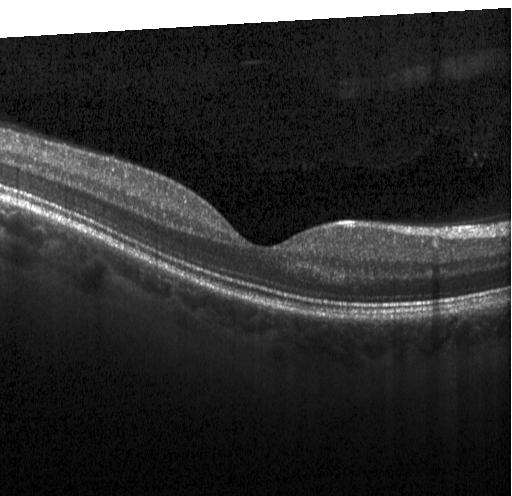
Finding: no choroidal neovascularization, no diabetic macular edema, and no drusen.